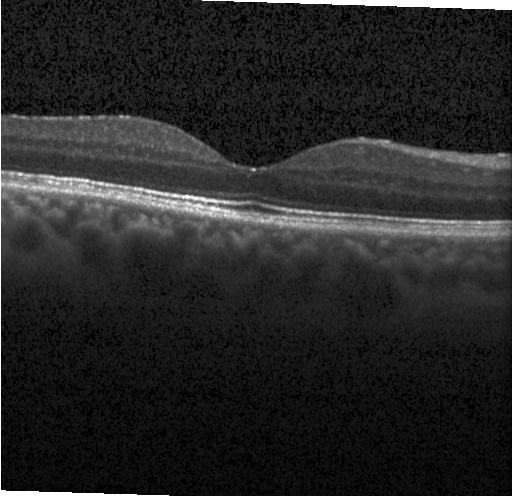

Retinal OCT B-scan. Instrument: Heidelberg Spectralis. SD-OCT. Dx: neither CNV, DME, nor drusen.